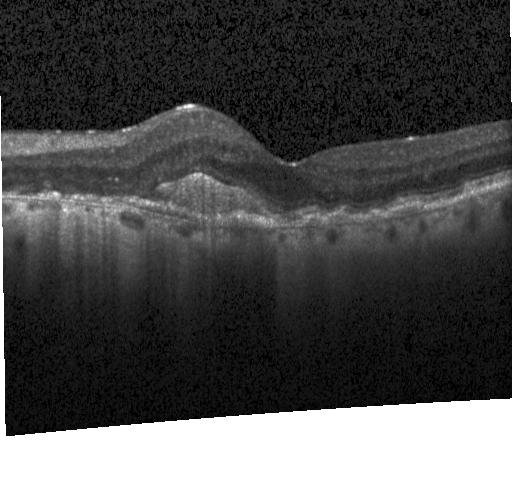
OCT scan showing CNV.